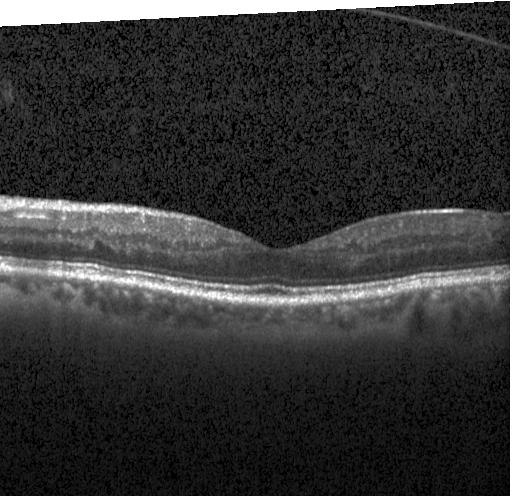
Retinal OCT B-scan — Impression: no choroidal neovascularization, no diabetic macular edema, and no drusen.